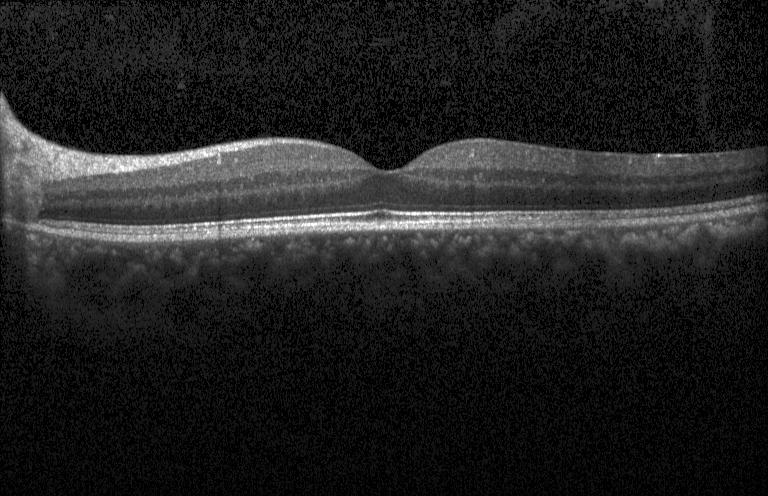

No choroidal neovascularization, diabetic macular edema, or drusen.